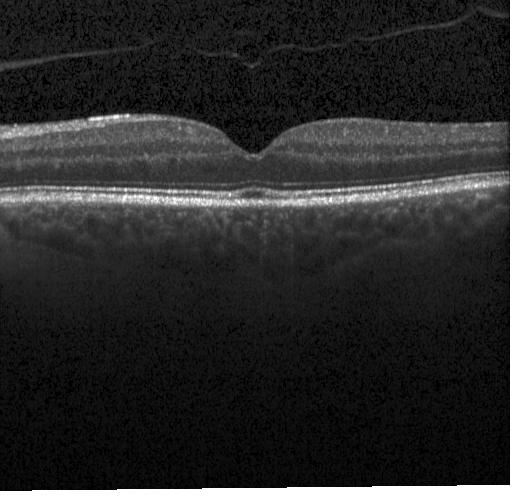 Macular OCT: no evidence of choroidal neovascularization, diabetic macular edema, or drusen.